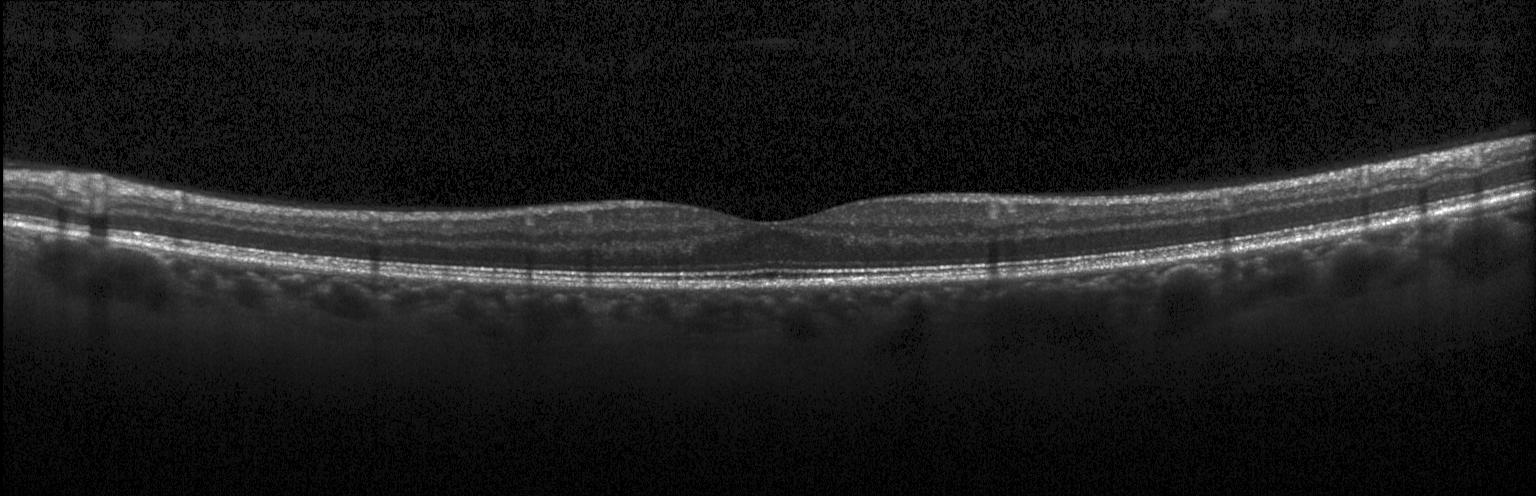 Finding: no choroidal neovascularization, diabetic macular edema, or drusen.